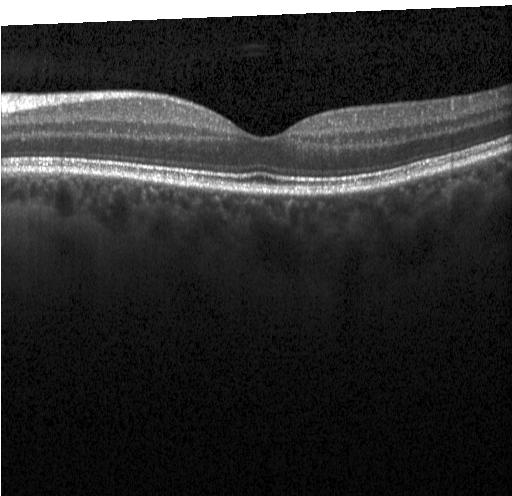 Spectral-domain optical coherence tomography · Heidelberg Spectralis · retinal OCT B-scan.
This B-scan demonstrates no choroidal neovascularization, no diabetic macular edema, and no drusen.